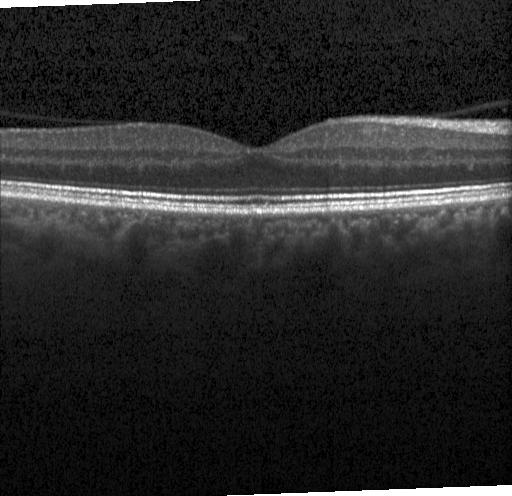
Optical coherence tomography B-scan; spectral-domain OCT; Heidelberg Spectralis. Impression: no evidence of choroidal neovascularization, diabetic macular edema, or drusen.